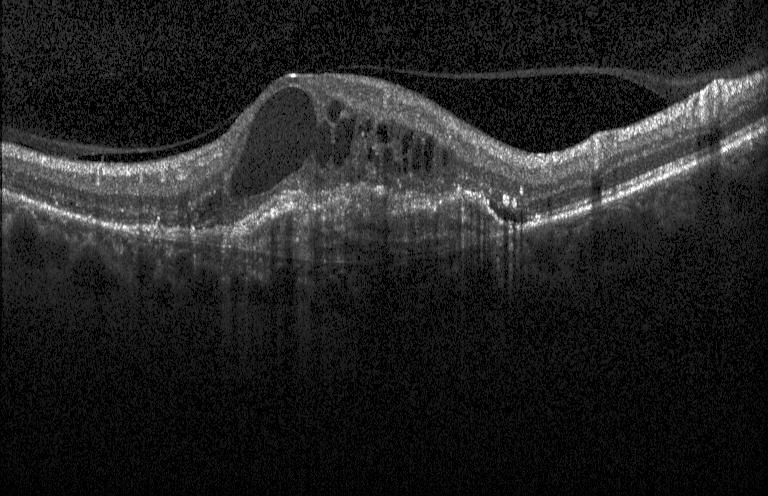

Finding: CNV.